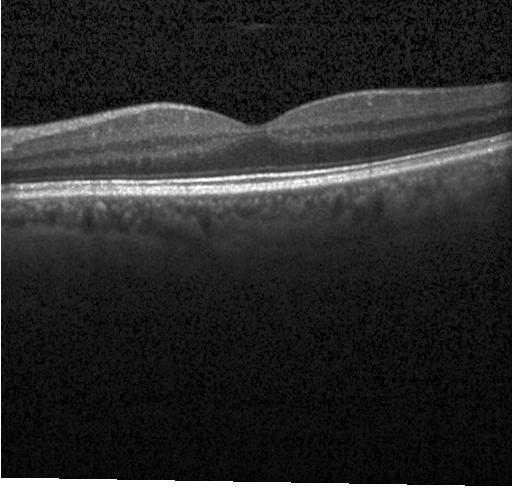 Spectral-domain OCT. Macular scan. OCT line scan. Assessment: no evidence of choroidal neovascularization, diabetic macular edema, or drusen.